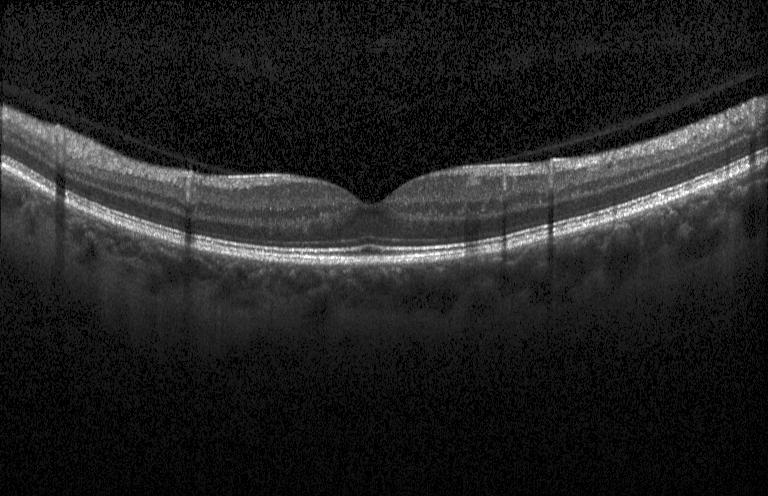
Spectral-domain OCT · horizontal scan through the fovea · OCT line scan — OCT finding: no CNV, no DME, and no drusen.